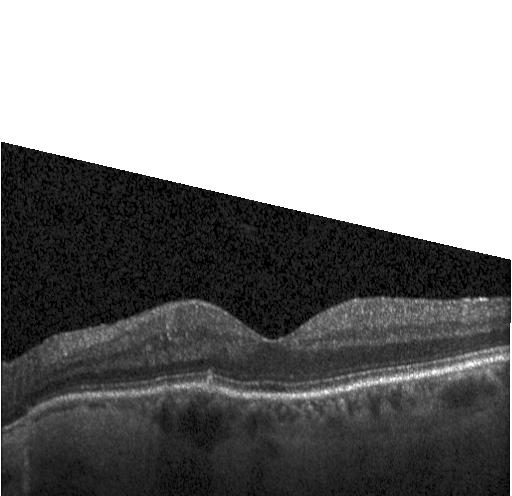
Instrument: Heidelberg Spectralis; OCT B-scan. This B-scan demonstrates multiple drusen.